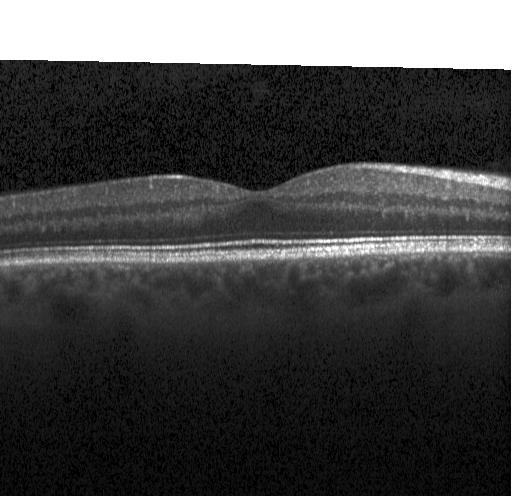 Spectral-domain OCT; horizontal scan through the fovea; Heidelberg Spectralis OCT system; OCT line scan
Assessment: no choroidal neovascularization, diabetic macular edema, or drusen.